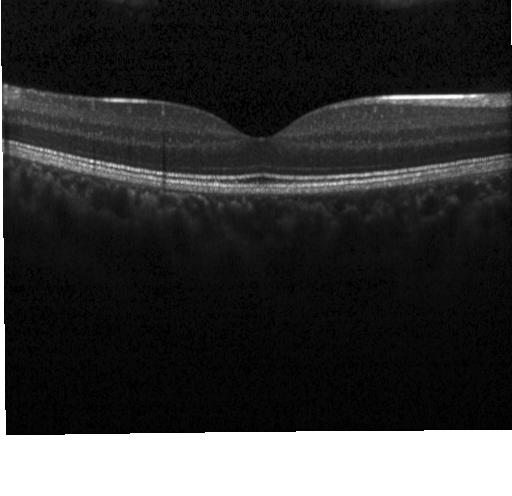 SD-OCT · retinal OCT B-scan
Impression: no choroidal neovascularization, diabetic macular edema, or drusen.